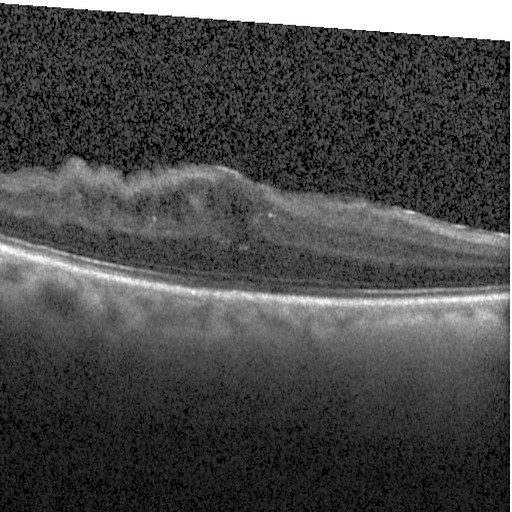

Finding: DME.